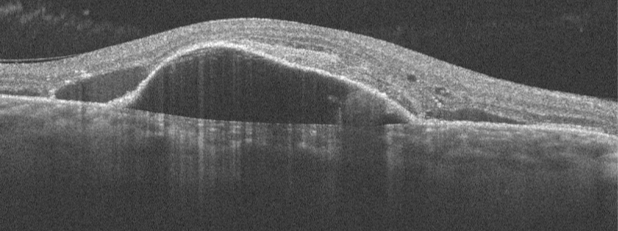

Impression: AMD.